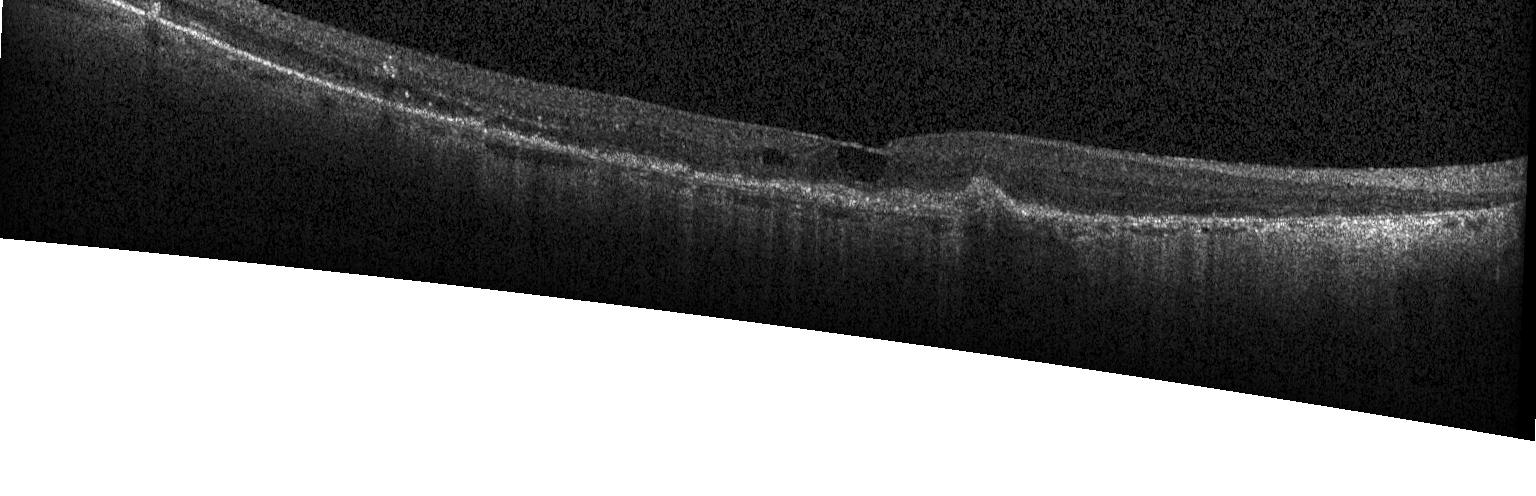
Acquired on a Heidelberg Spectralis; optical coherence tomography scan; SD-OCT — This B-scan demonstrates a choroidal neovascular membrane.